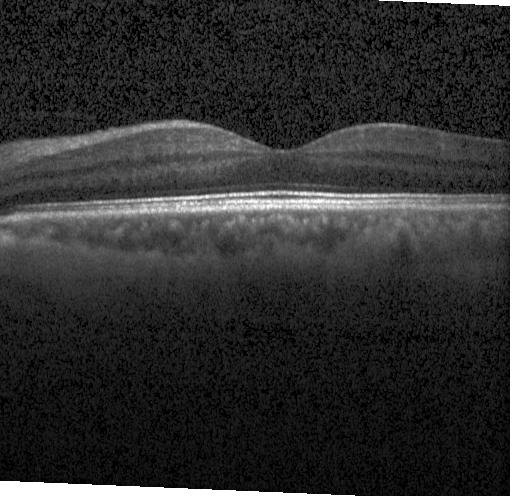 OCT scan showing no CNV, DME, or drusen.